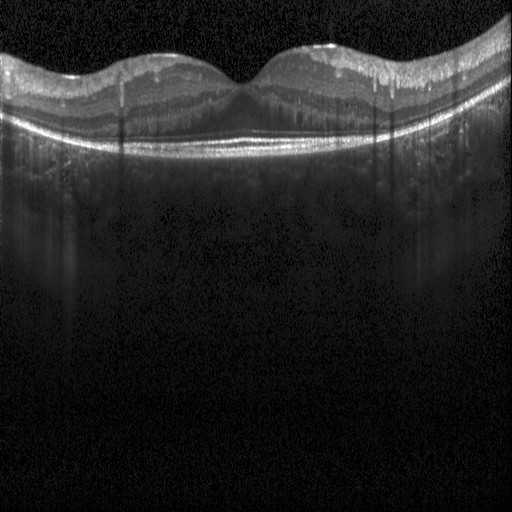 Spectral-domain OCT. OCT B-scan.
Finding: diabetic macular edema.